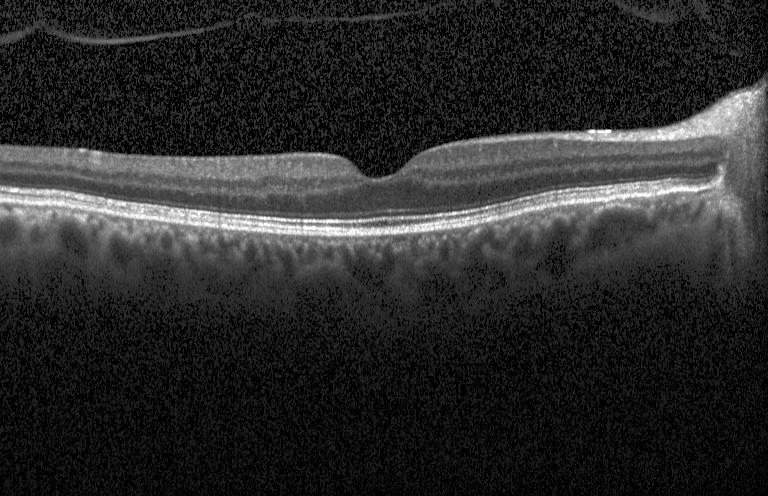
Acquired on a Heidelberg Spectralis, optical coherence tomography B-scan, spectral-domain optical coherence tomography, through the macula. This B-scan demonstrates no evidence of CNV, DME, or drusen.